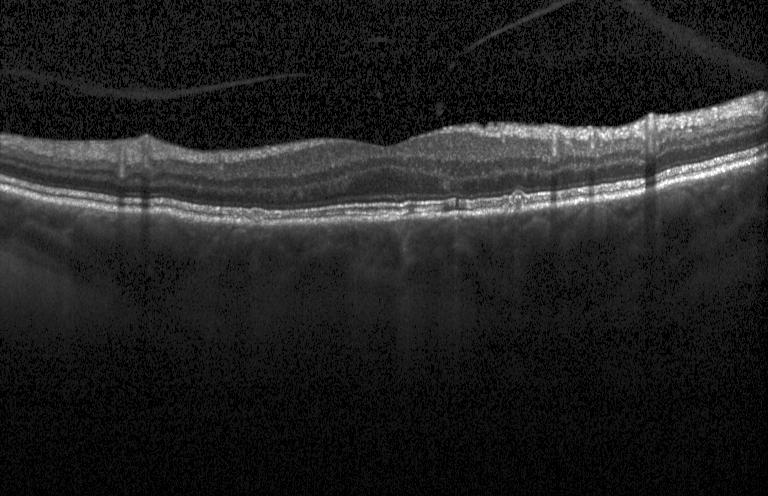
Diagnosis: multiple drusen.